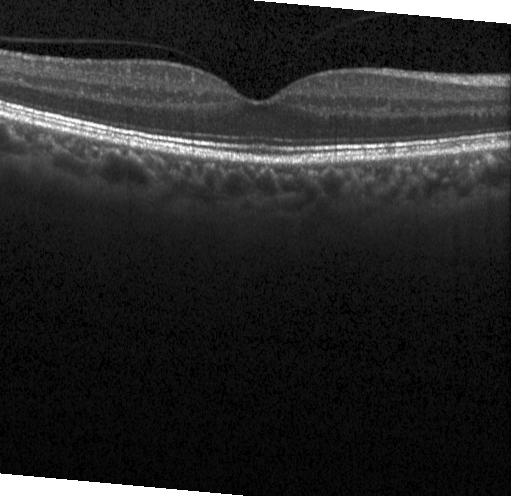

Assessment: no choroidal neovascularization, no diabetic macular edema, and no drusen.